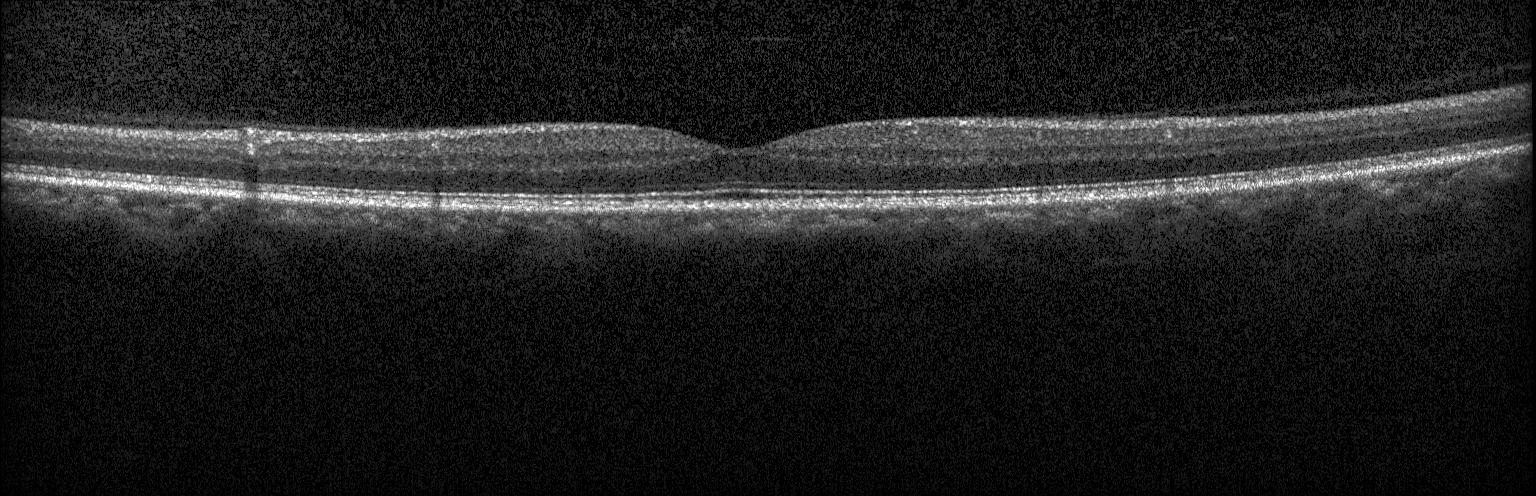 Macular scan. Retinal OCT cross-section. Spectral-domain optical coherence tomography. Impression: neither choroidal neovascularization, diabetic macular edema, nor drusen.